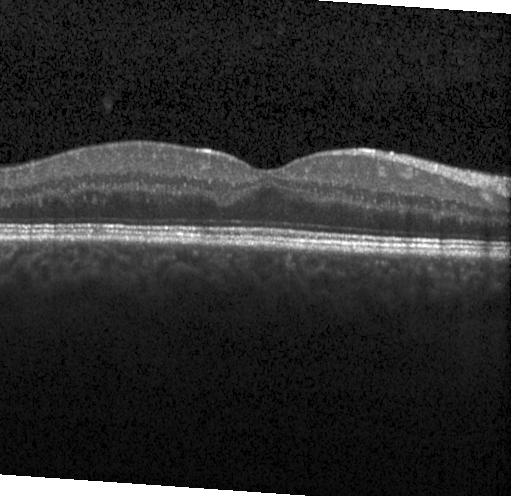

Optical coherence tomography B-scan
No evidence of CNV, DME, or drusen.